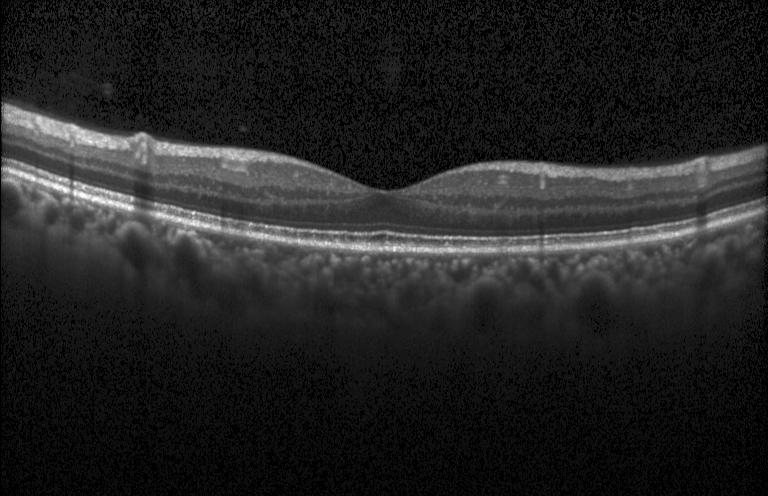

The scan shows neither CNV, DME, nor drusen.